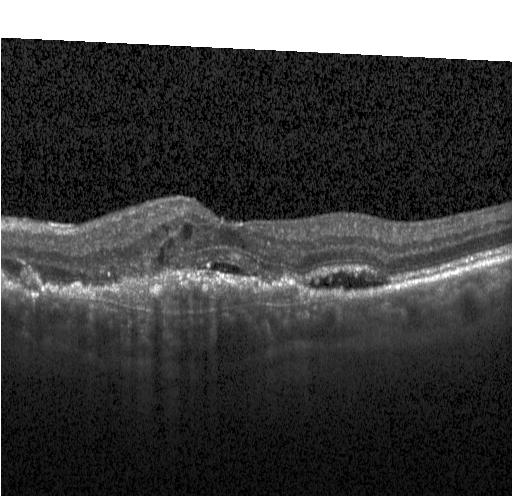

OCT line scan — Impression: CNV.